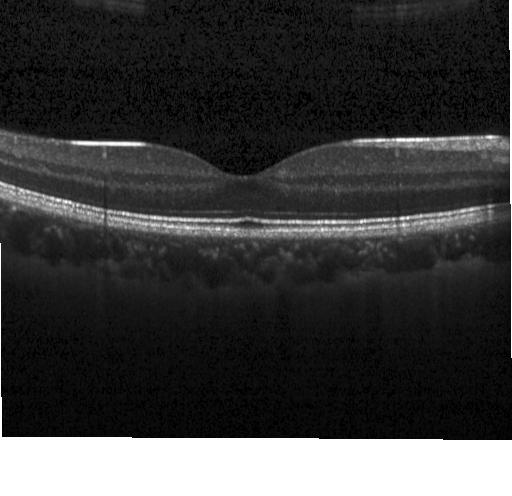
Macular OCT demonstrating neither CNV, DME, nor drusen.